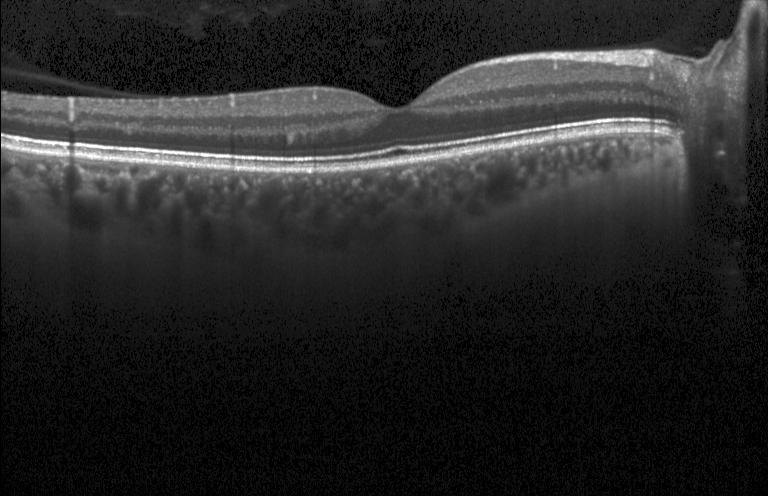

Centered on the fovea, SD-OCT, retinal OCT B-scan.
Impression: no choroidal neovascularization, no diabetic macular edema, and no drusen.